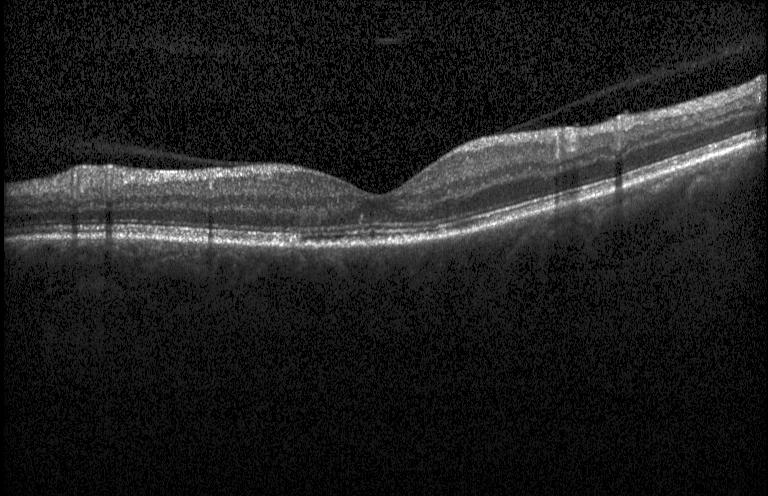

OCT line scan
Macular OCT: no evidence of CNV, DME, or drusen.